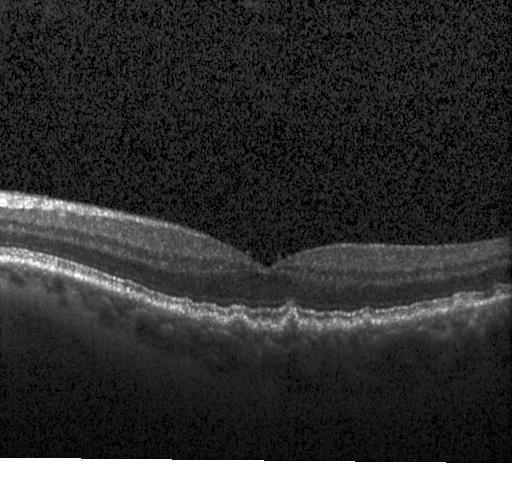 Spectral-domain OCT · acquired on a Heidelberg Spectralis · optical coherence tomography scan. Dx: drusen.